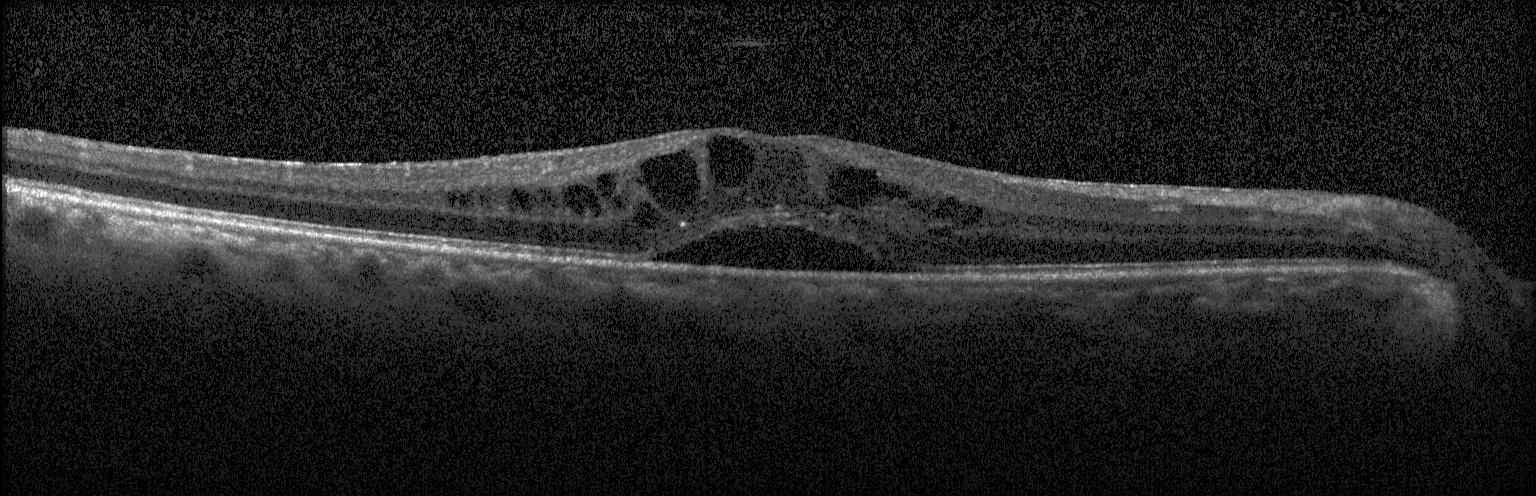
OCT line scan. OCT finding: diabetic macular edema (DME).